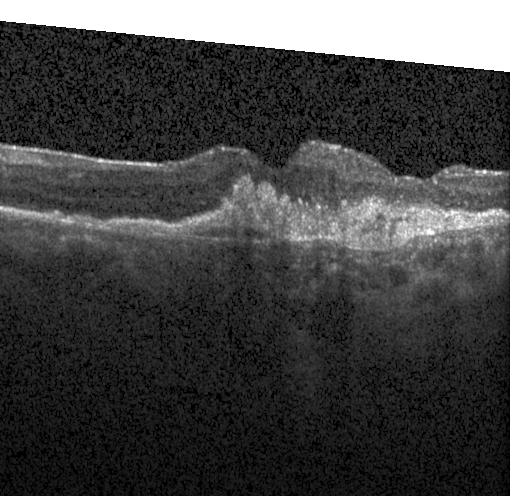 OCT line scan; Heidelberg Spectralis — Assessment: CNV.